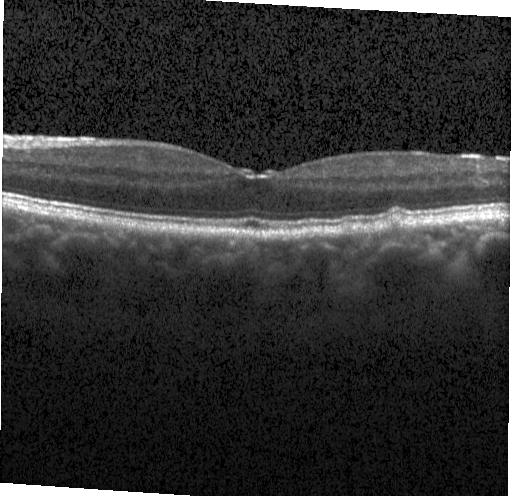
Optical coherence tomography B-scan — Finding: multiple drusen.